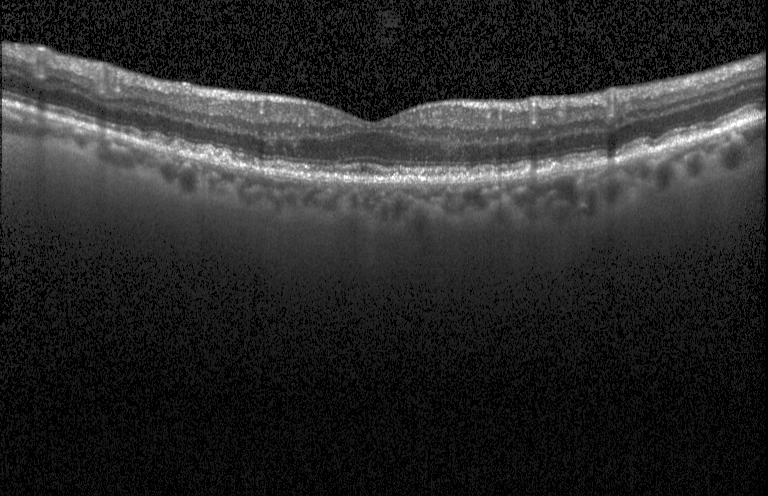

Fovea-centered; OCT line scan; Heidelberg Spectralis; SD-OCT. Diagnosis: sub-RPE drusenoid deposits.